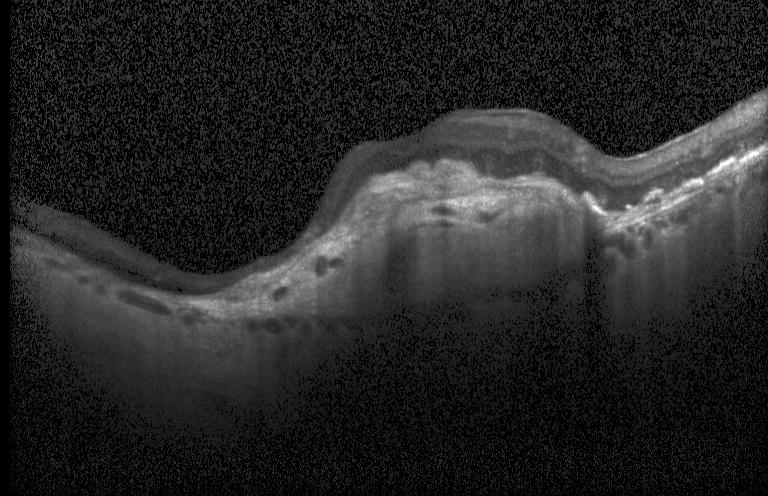 Optical coherence tomography scan
Macular OCT: a choroidal neovascular membrane.